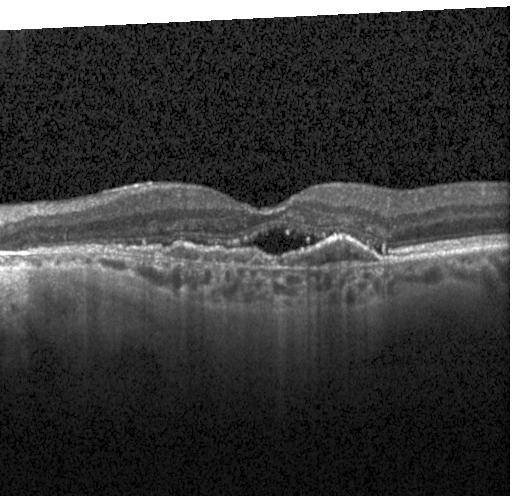
OCT B-scan, Heidelberg Spectralis OCT system, SD-OCT, fovea-centered — Impression: a choroidal neovascular membrane.